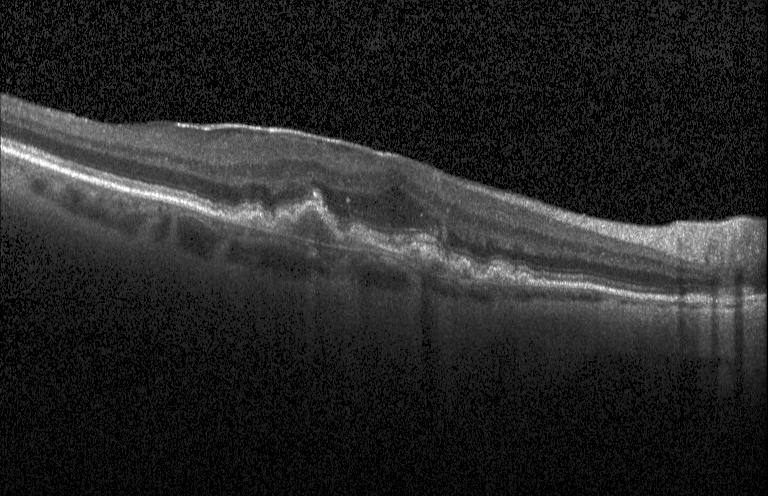

Impression: multiple drusen.